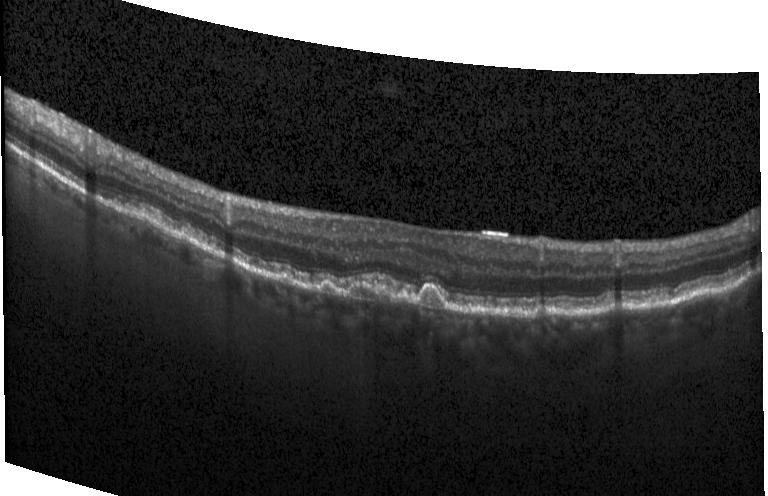 Impression: multiple drusen.